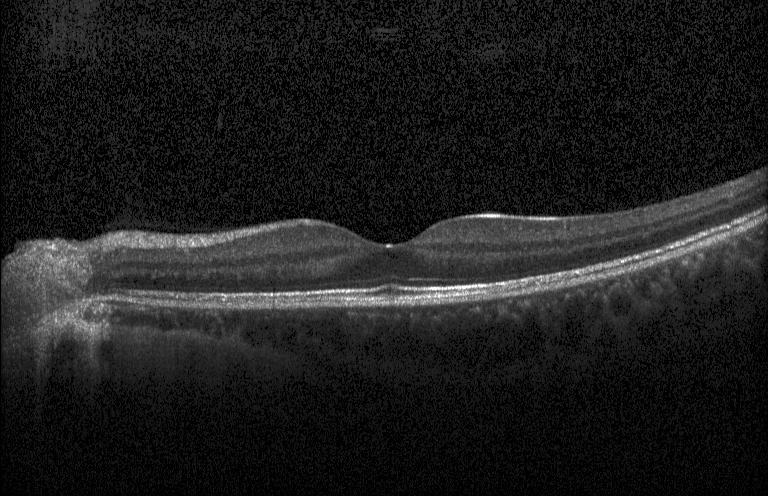
Spectral-domain OCT; Heidelberg Spectralis OCT system; optical coherence tomography scan; centered on the fovea.
Assessment: no evidence of CNV, DME, or drusen.